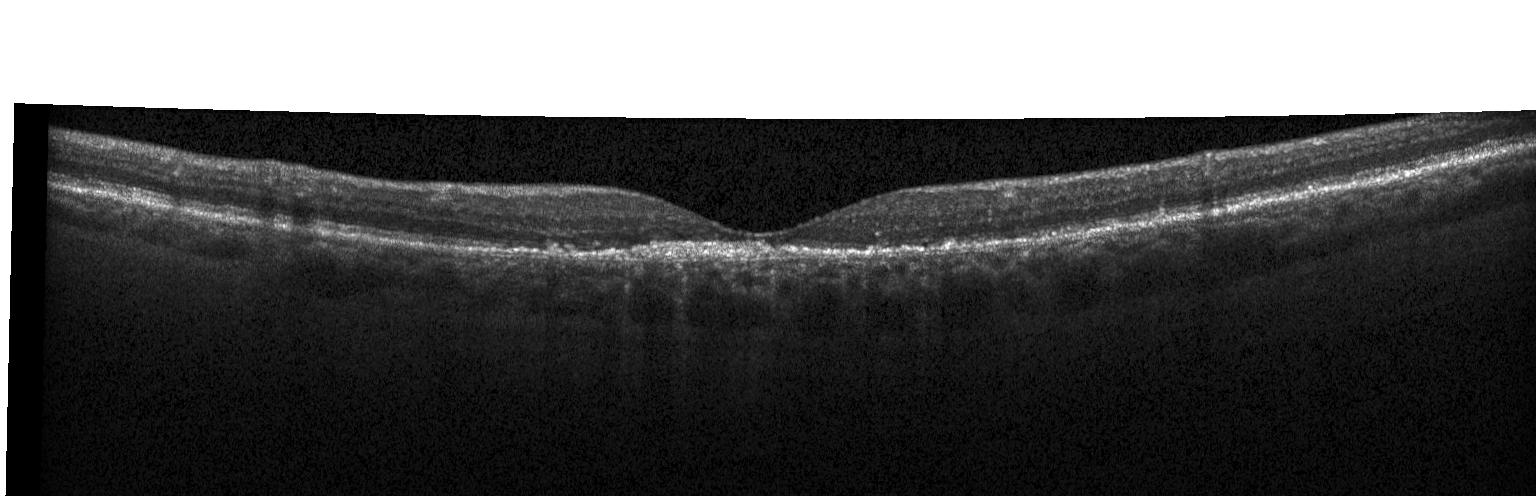
Retinal OCT cross-section — Diagnosis: a choroidal neovascular membrane.